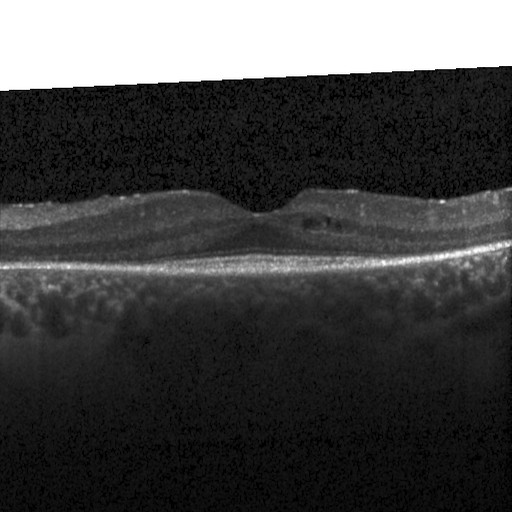
OCT B-scan. Finding: DME.